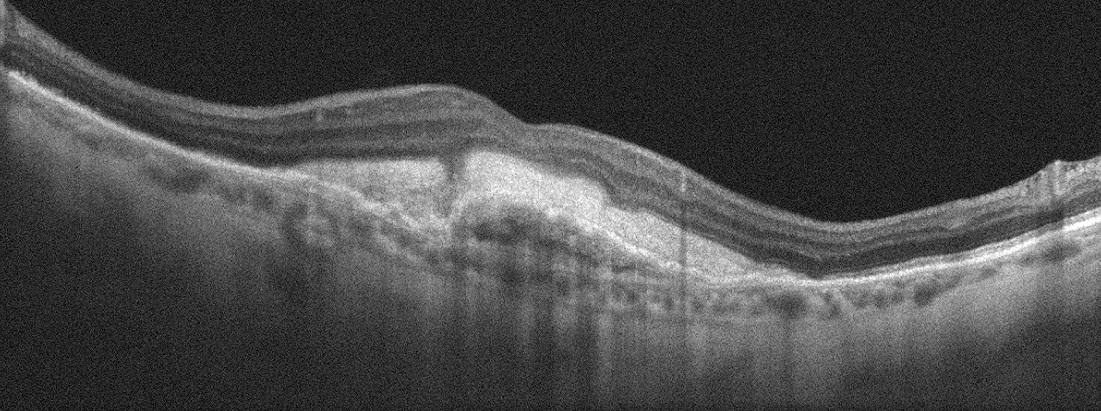 Finding: age-related macular degeneration.